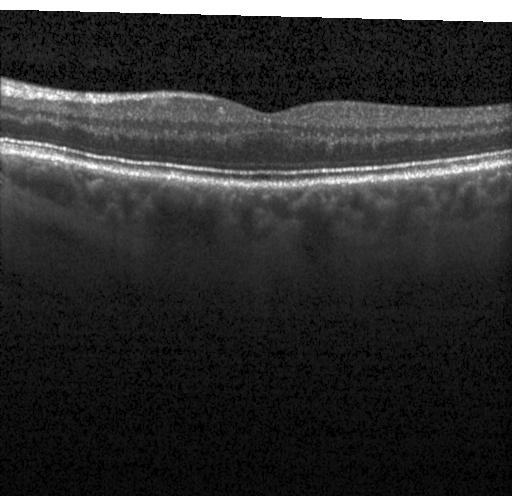 Retinal OCT cross-section showing no choroidal neovascularization, diabetic macular edema, or drusen.